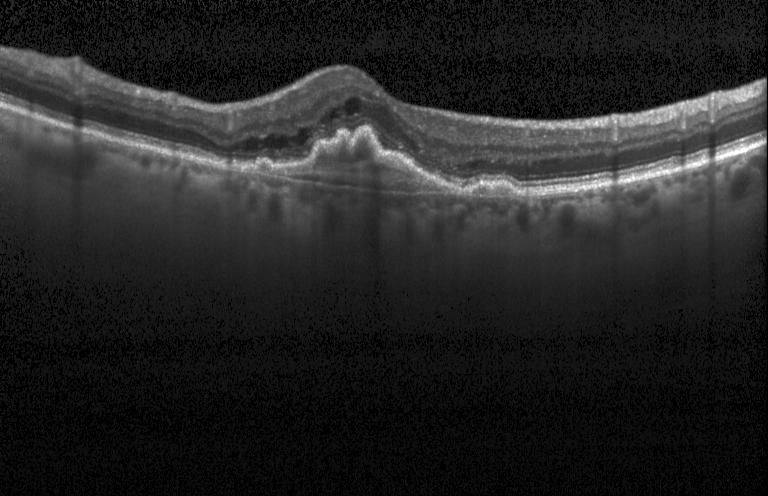 SD-OCT, retinal OCT cross-section, Heidelberg Spectralis, centered on the fovea.
Assessment: a choroidal neovascular membrane.